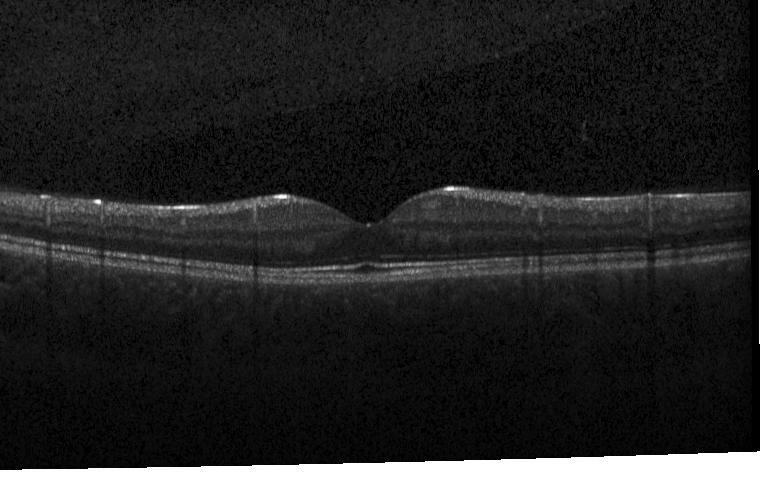

Instrument: Heidelberg Spectralis, OCT B-scan, spectral-domain optical coherence tomography — Neither CNV, DME, nor drusen.